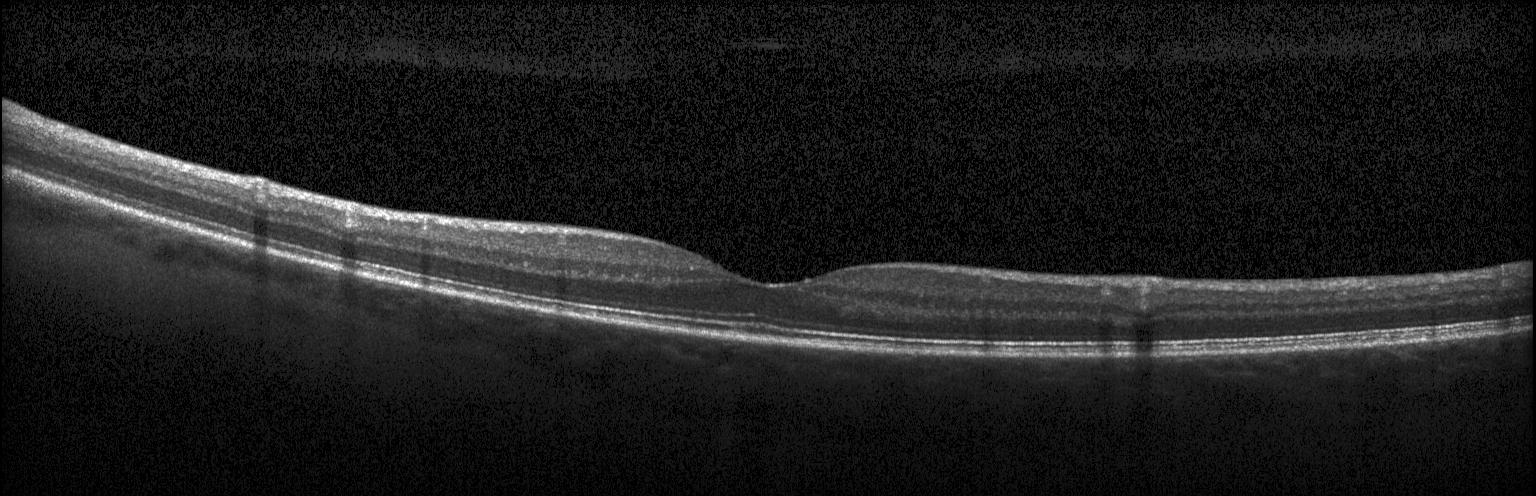
Spectral-domain OCT, retinal OCT B-scan
Finding: neither choroidal neovascularization, diabetic macular edema, nor drusen.